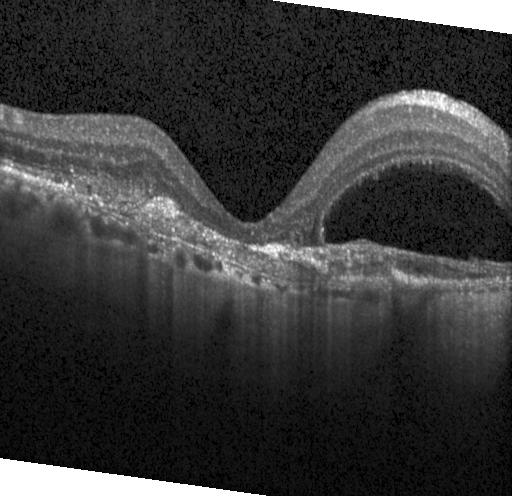

Optical coherence tomography scan. Instrument: Heidelberg Spectralis.
Diagnosis: a choroidal neovascular membrane.